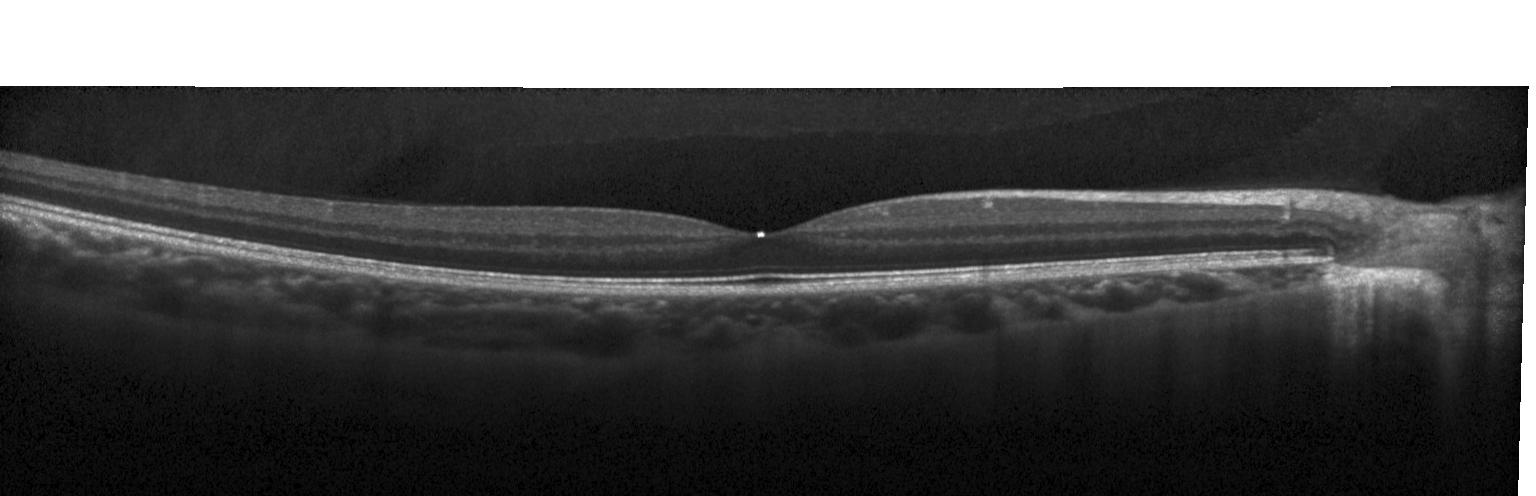
Spectral-domain optical coherence tomography. OCT line scan. Through the macula. Heidelberg Spectralis OCT system — Impression: no choroidal neovascularization, no diabetic macular edema, and no drusen.